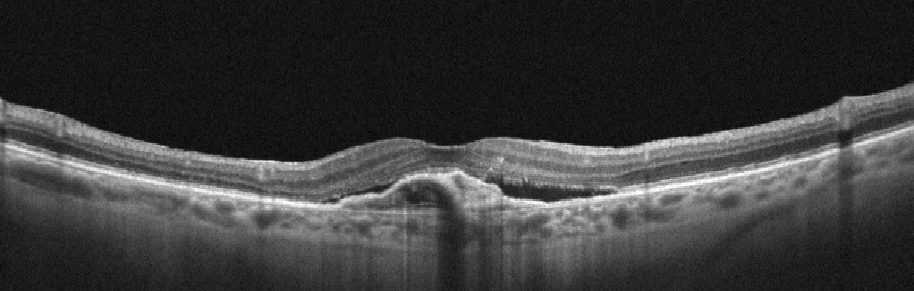

Diagnosis: age-related macular degeneration (AMD).